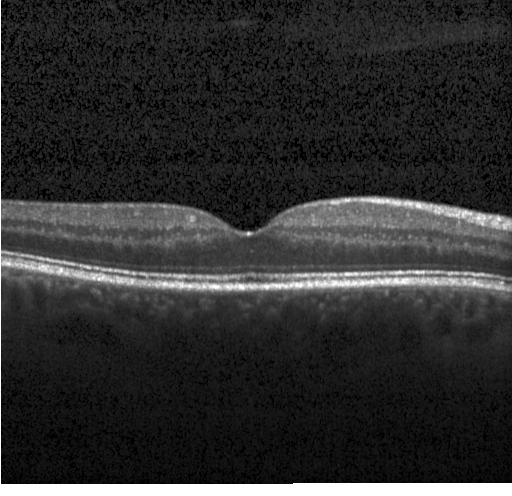 Finding: no evidence of choroidal neovascularization, diabetic macular edema, or drusen.